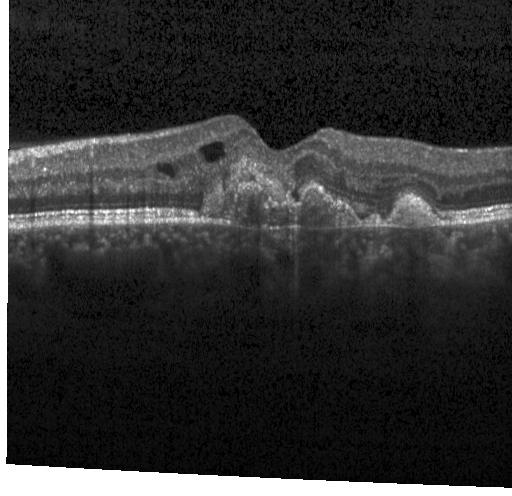

Impression: a choroidal neovascular membrane.